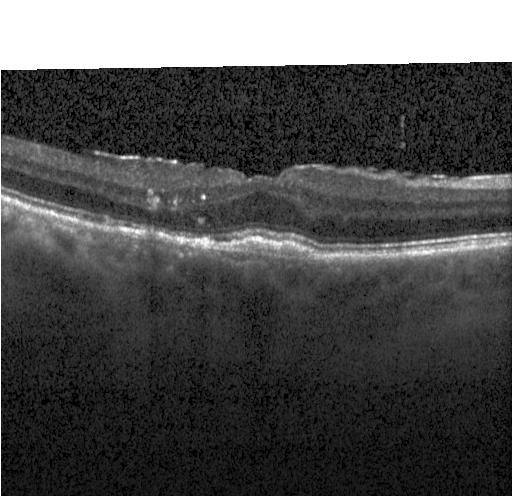
Impression: choroidal neovascularization (CNV).